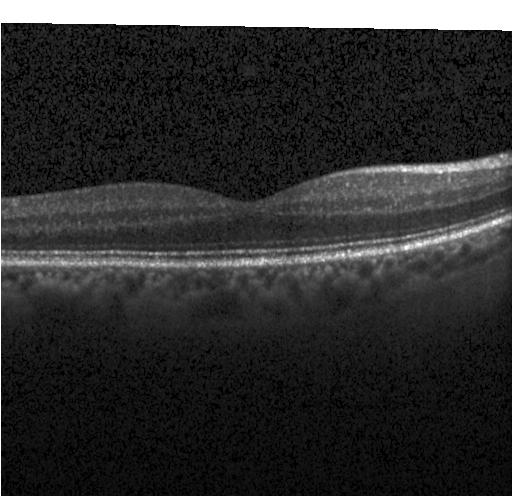 Macular OCT demonstrating no choroidal neovascularization, no diabetic macular edema, and no drusen.